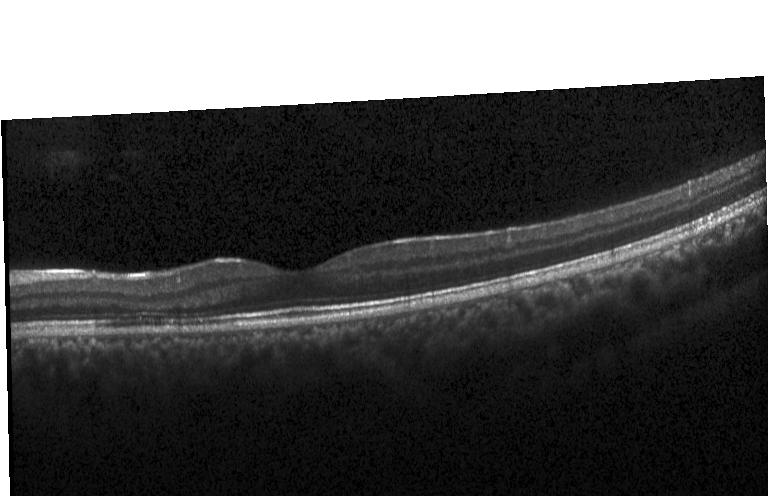

Finding: no CNV, no DME, and no drusen.